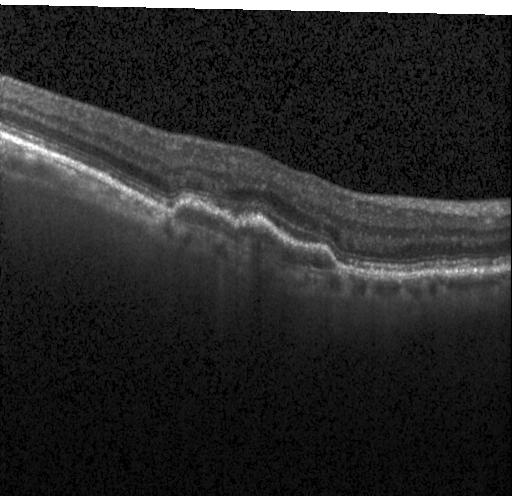
Optical coherence tomography scan, SD-OCT, instrument: Heidelberg Spectralis. Diagnosis: choroidal neovascularization.